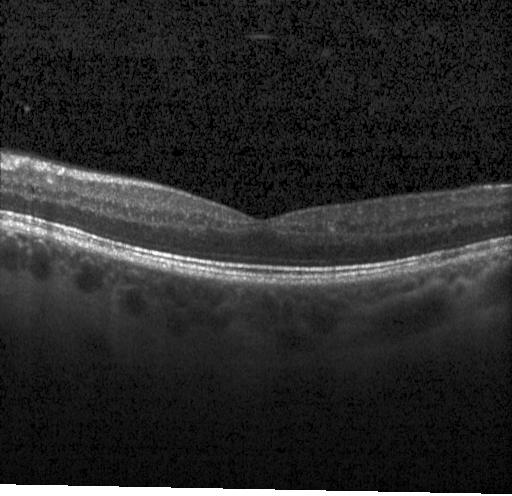

OCT finding: no CNV, no DME, and no drusen.